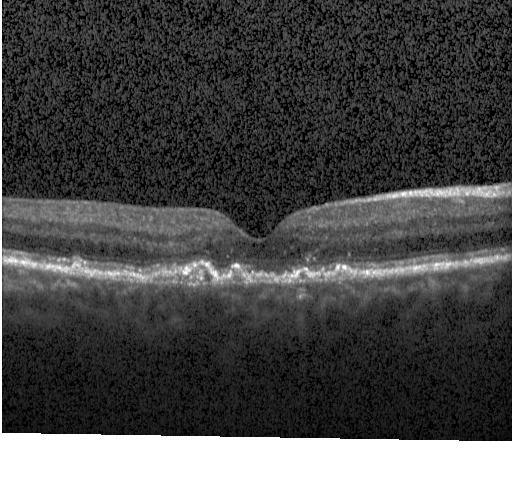
Retinal OCT cross-section. Finding: choroidal neovascularization.